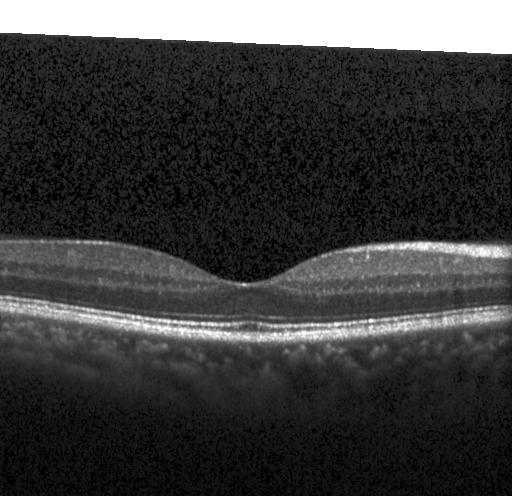

OCT line scan; instrument: Heidelberg Spectralis
Diagnosis: no choroidal neovascularization, diabetic macular edema, or drusen.